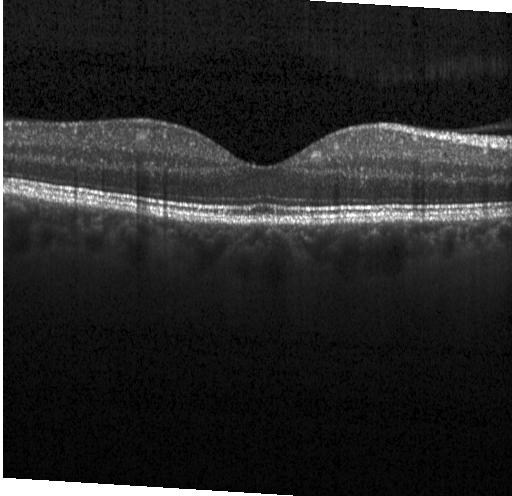

Impression: neither choroidal neovascularization, diabetic macular edema, nor drusen.